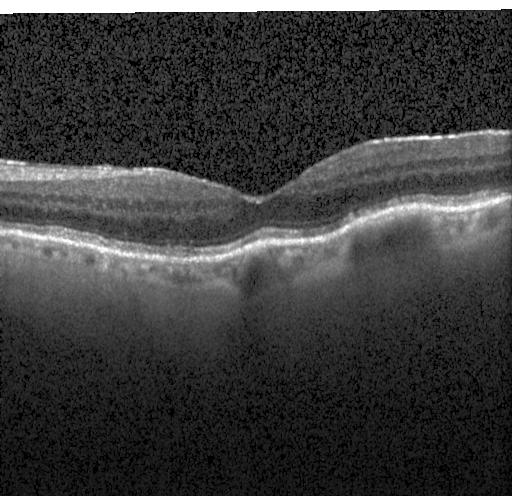 Dx: neither choroidal neovascularization, diabetic macular edema, nor drusen.